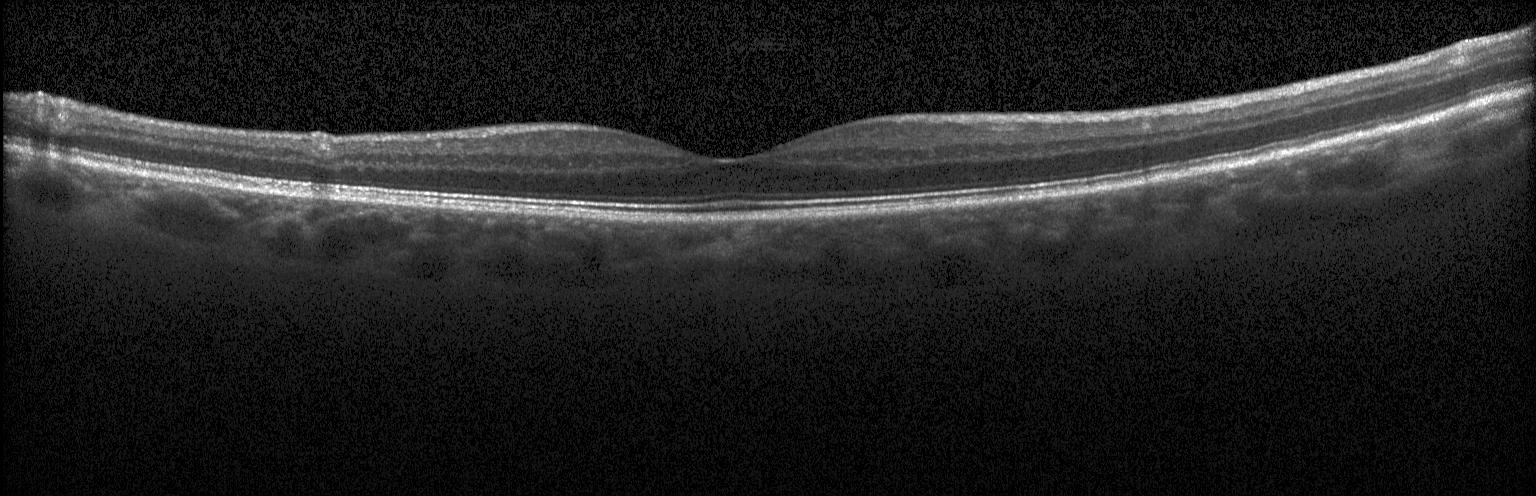

Dx: no evidence of choroidal neovascularization, diabetic macular edema, or drusen.